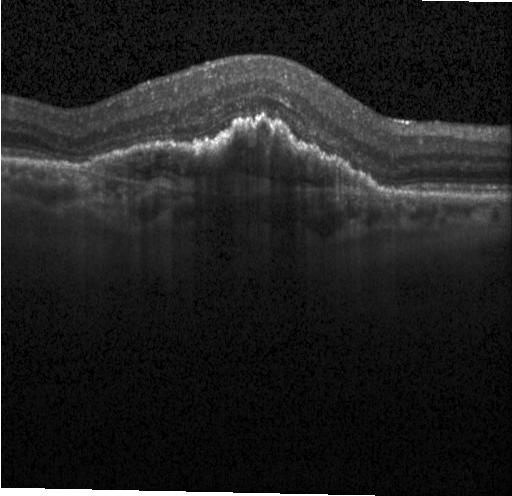
Dx: a choroidal neovascular membrane.